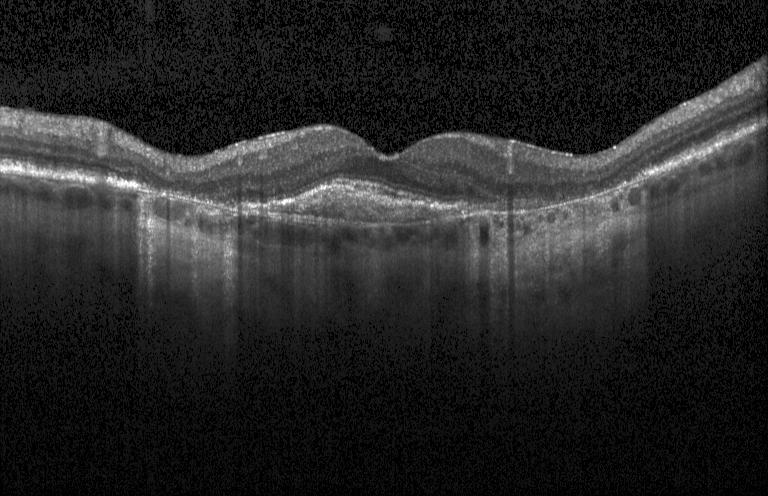
Finding: a choroidal neovascular membrane.